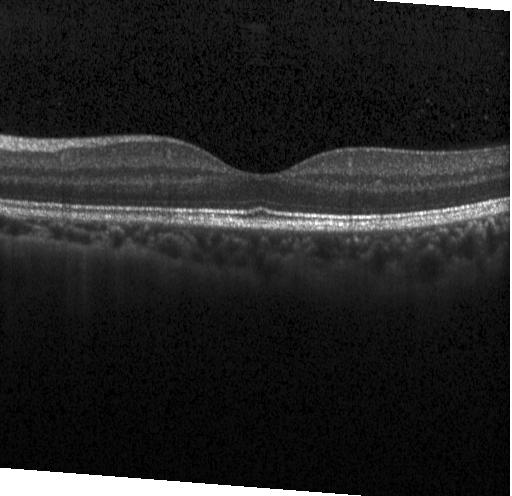

Finding: no evidence of choroidal neovascularization, diabetic macular edema, or drusen.